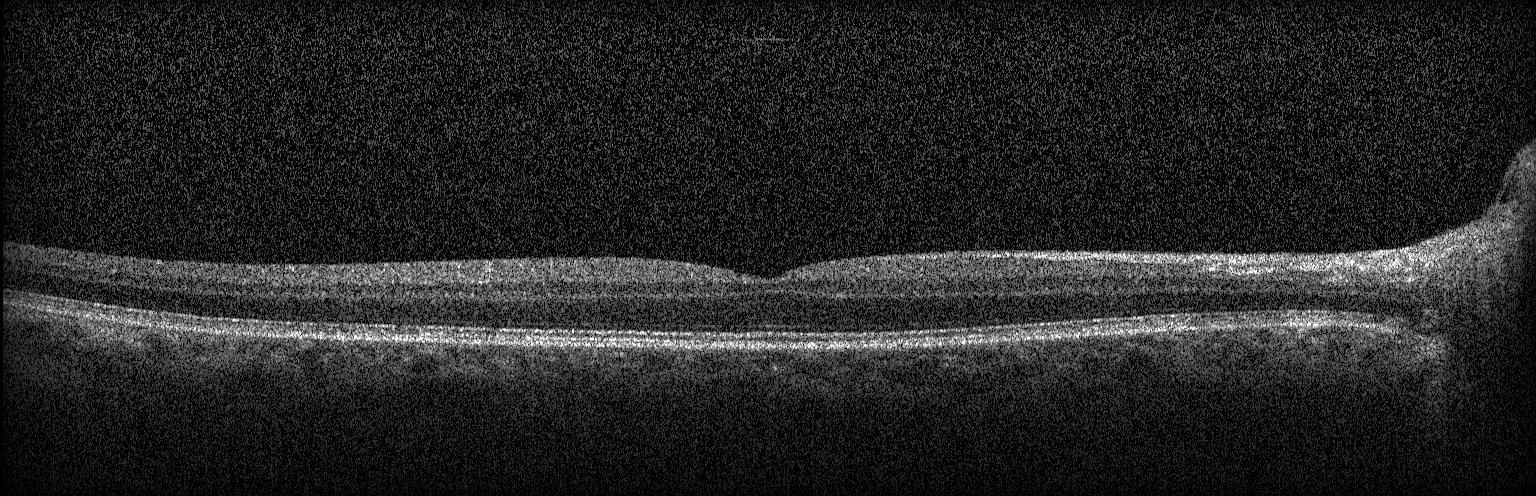
No evidence of choroidal neovascularization, diabetic macular edema, or drusen.